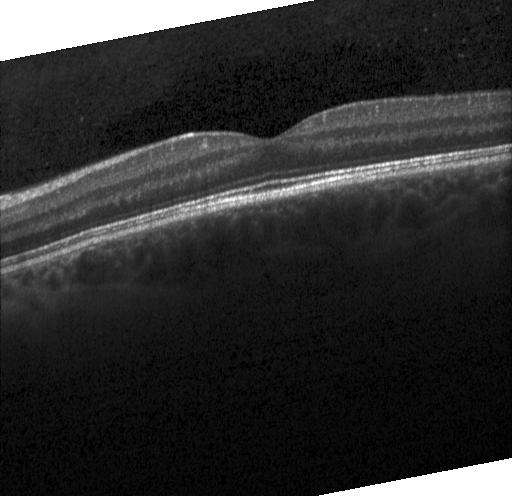
Impression: no evidence of CNV, DME, or drusen.